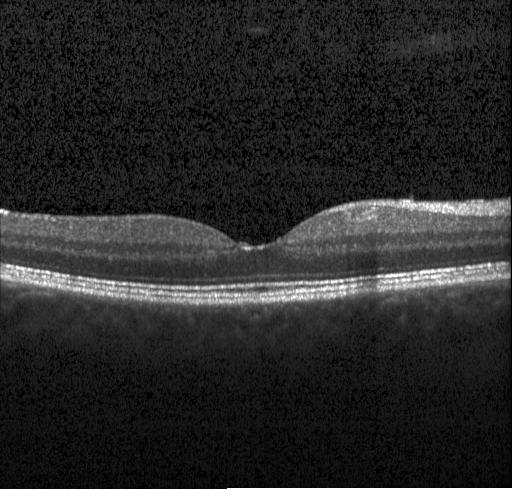
Instrument: Heidelberg Spectralis, through the macula, OCT B-scan, SD-OCT. Diagnosis: no choroidal neovascularization, no diabetic macular edema, and no drusen.